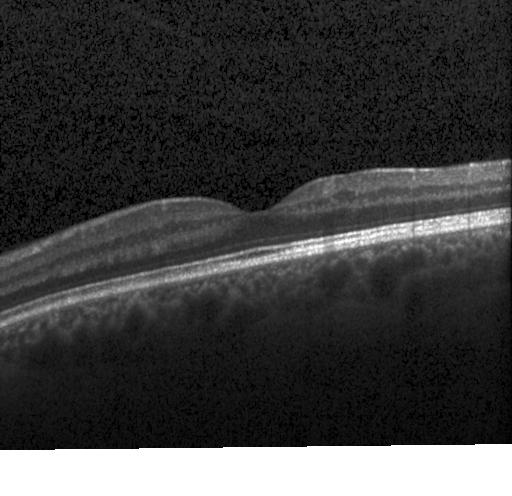 Spectral-domain OCT B-scan: no choroidal neovascularization, no diabetic macular edema, and no drusen.